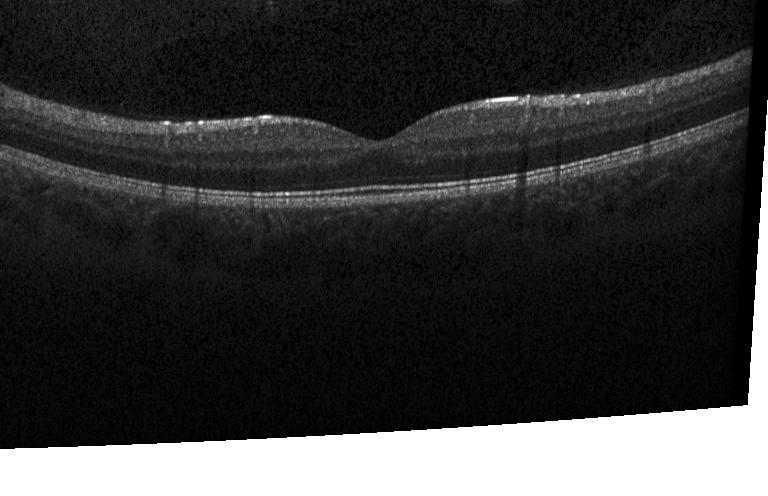

Horizontal scan through the fovea. SD-OCT. Heidelberg Spectralis OCT system. Retinal OCT cross-section.
Diagnosis: no evidence of CNV, DME, or drusen.